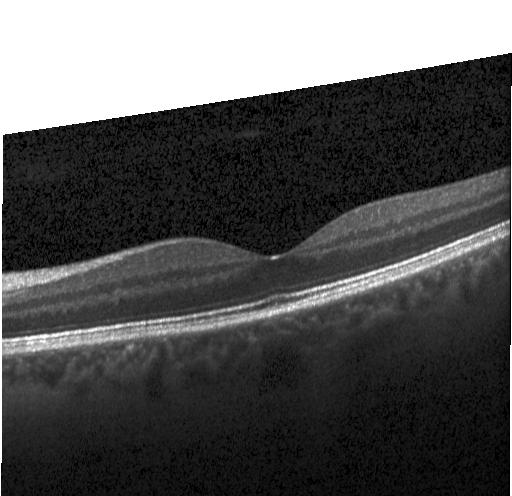 Fovea-centered, optical coherence tomography scan
The scan shows no evidence of choroidal neovascularization, diabetic macular edema, or drusen.